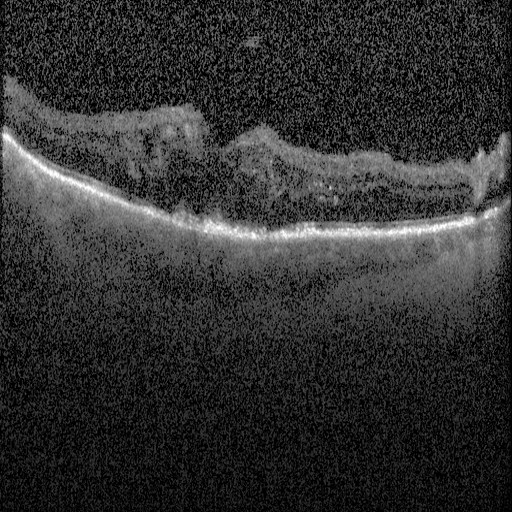

DME.